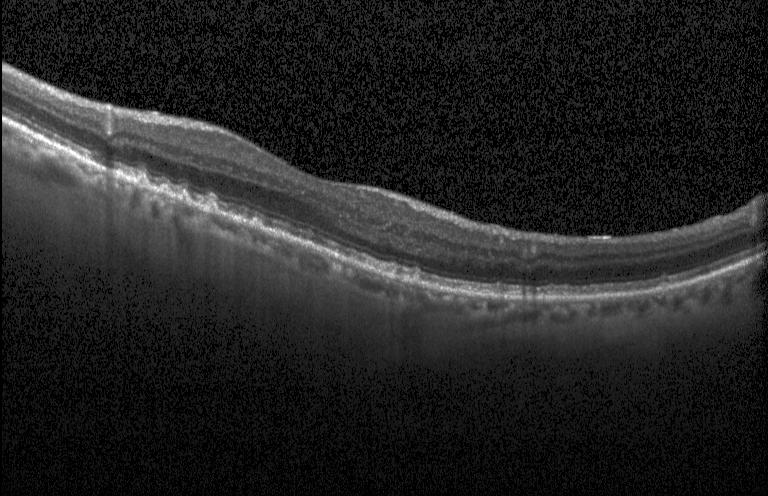
Optical coherence tomography B-scan.
Finding: sub-RPE drusenoid deposits.